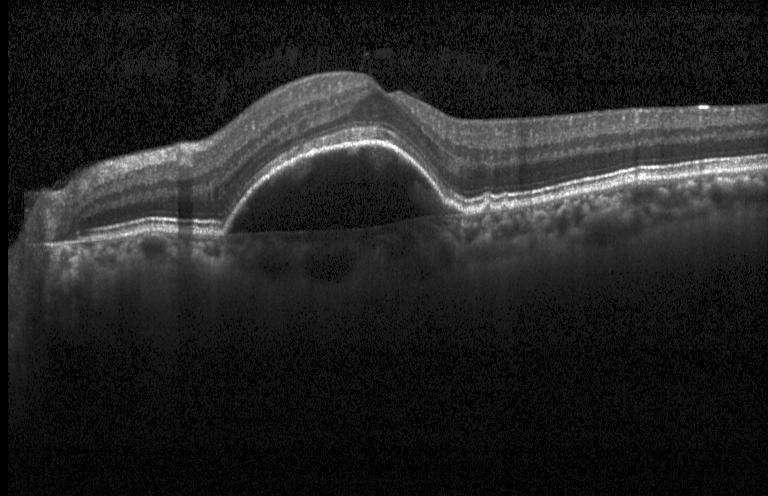 Impression: a choroidal neovascular membrane.